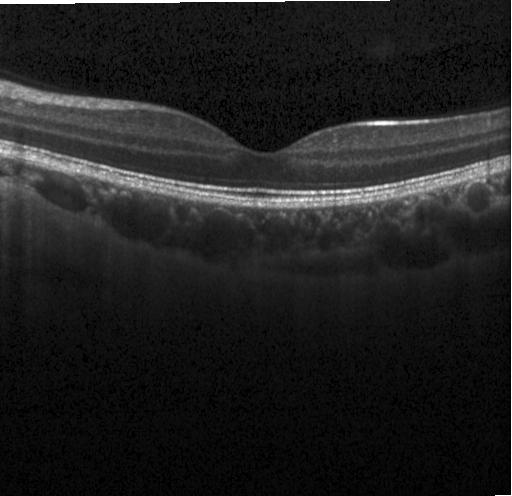
Retinal OCT cross-section, spectral-domain optical coherence tomography, acquired on a Heidelberg Spectralis — The scan shows no evidence of choroidal neovascularization, diabetic macular edema, or drusen.